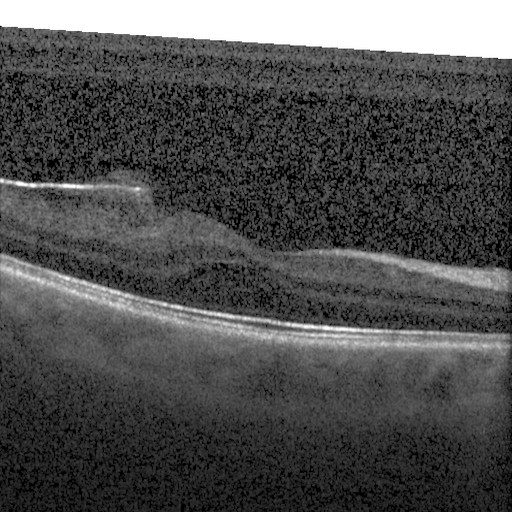 Heidelberg Spectralis · spectral-domain OCT · optical coherence tomography scan · fovea-centered — Finding: diabetic macular edema (DME).